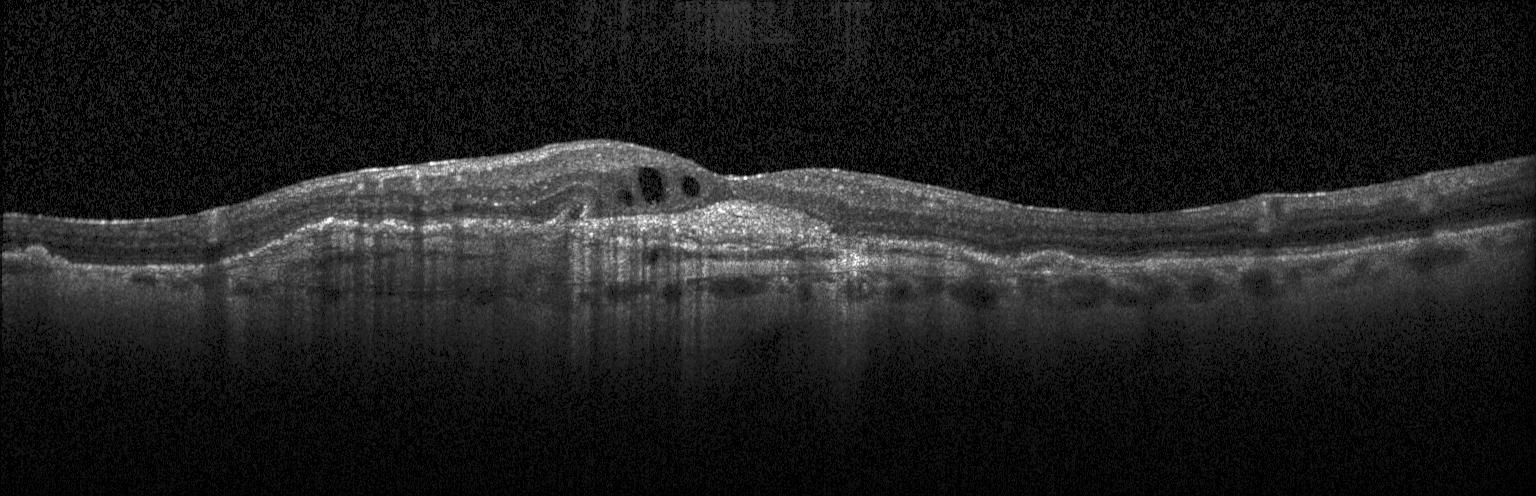
SD-OCT. OCT B-scan
Dx: choroidal neovascularization.